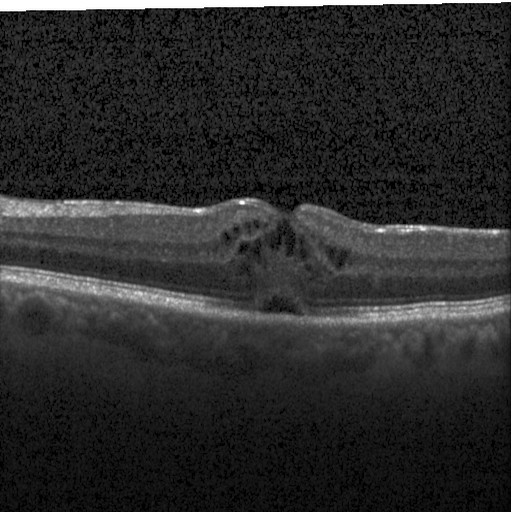
Impression: diabetic macular edema.